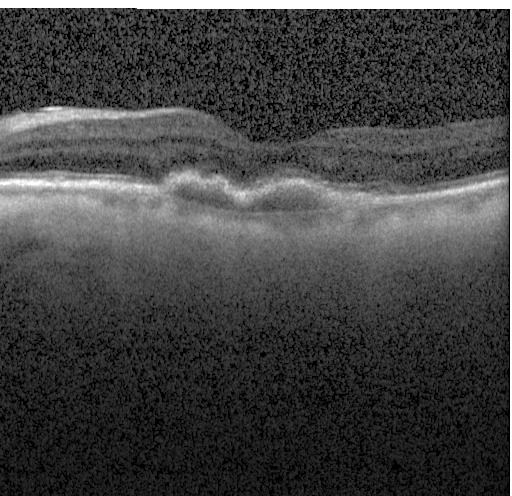 Finding: a choroidal neovascular membrane.